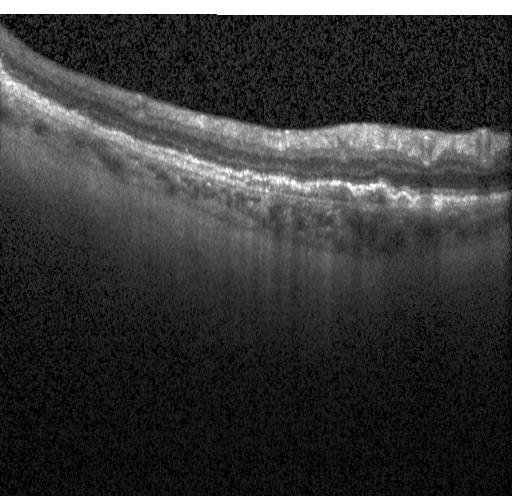 Retinal OCT cross-section · horizontal scan through the fovea.
Macular OCT: choroidal neovascularization (CNV).